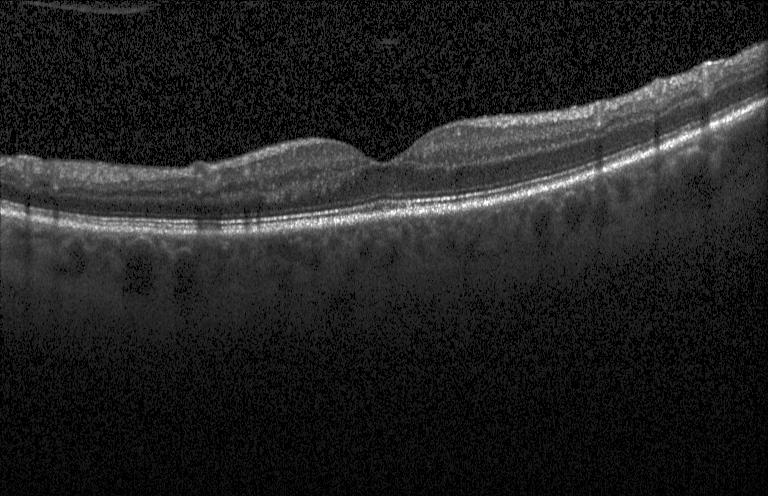 OCT B-scan — Diagnosis: neither choroidal neovascularization, diabetic macular edema, nor drusen.